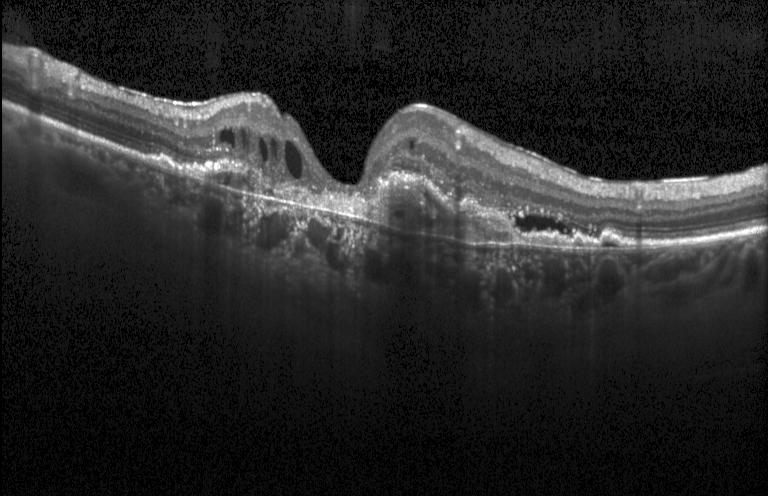 This B-scan demonstrates a choroidal neovascular membrane.